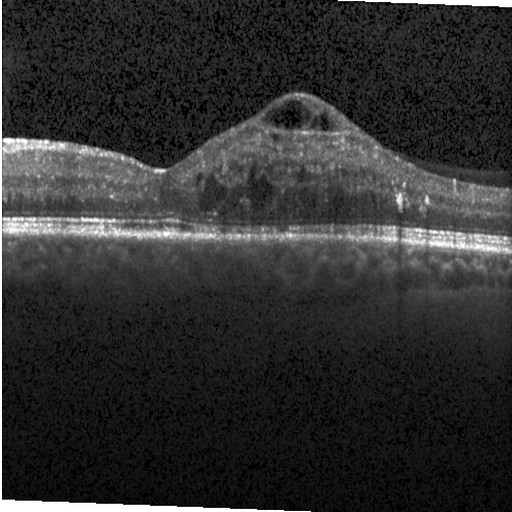

Heidelberg Spectralis OCT system · retinal OCT B-scan · SD-OCT · fovea-centered
Assessment: diabetic macular edema (DME).